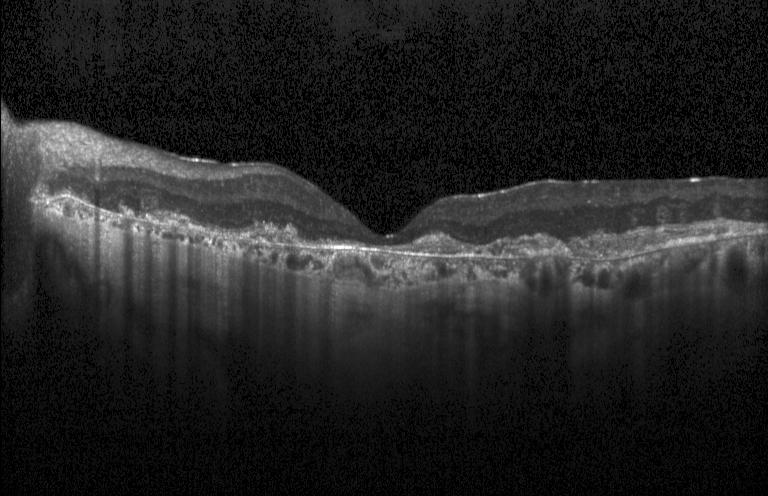
Retinal OCT cross-section showing a choroidal neovascular membrane.